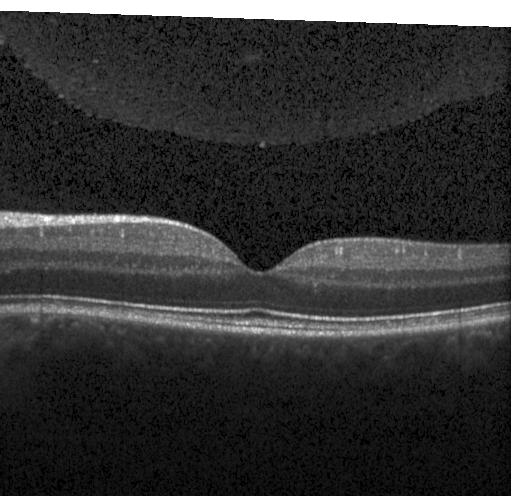 OCT B-scan showing no choroidal neovascularization, diabetic macular edema, or drusen.